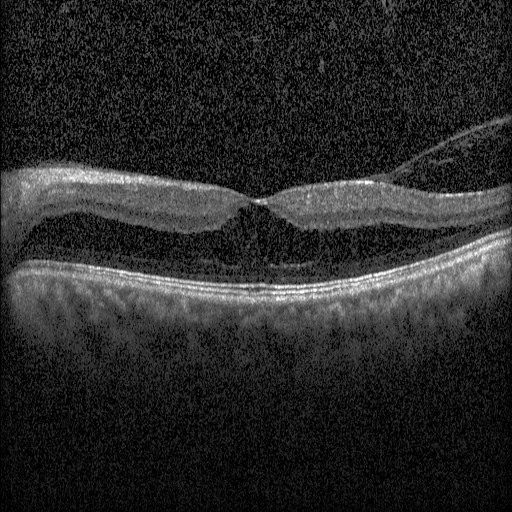 Dx: DME.